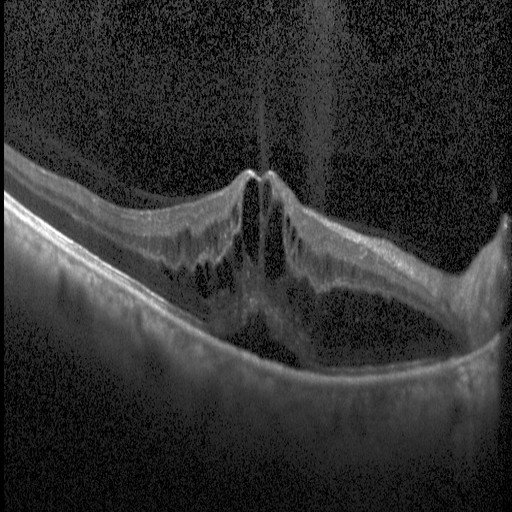 OCT B-scan, acquired on a Heidelberg Spectralis.
Assessment: DME.